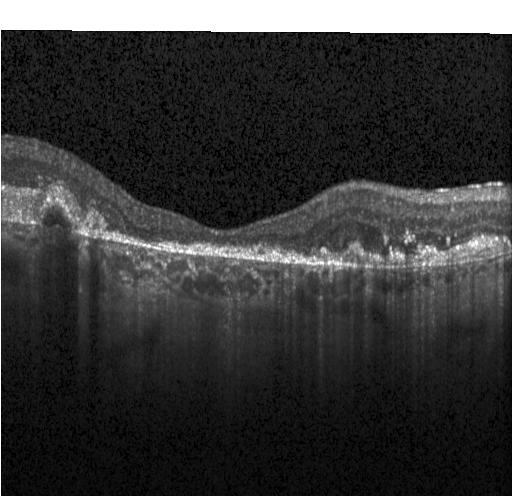
Spectral-domain OCT; retinal OCT B-scan; macular scan. Finding: choroidal neovascularization.